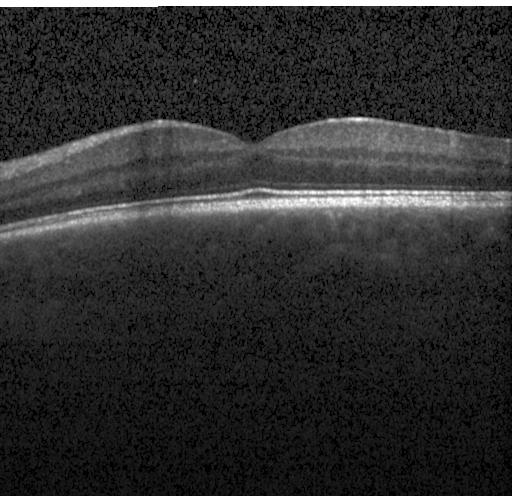 Impression: no CNV, DME, or drusen.